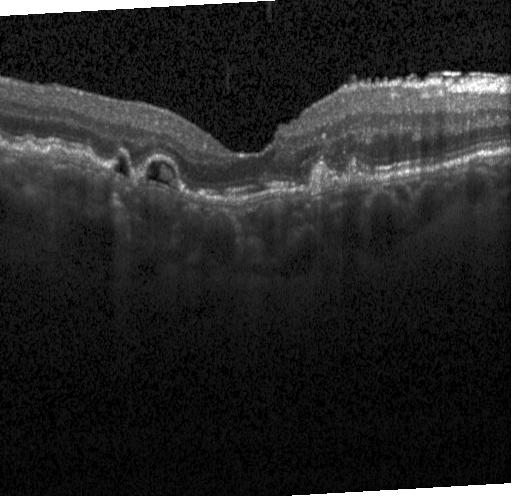

Finding: a choroidal neovascular membrane.